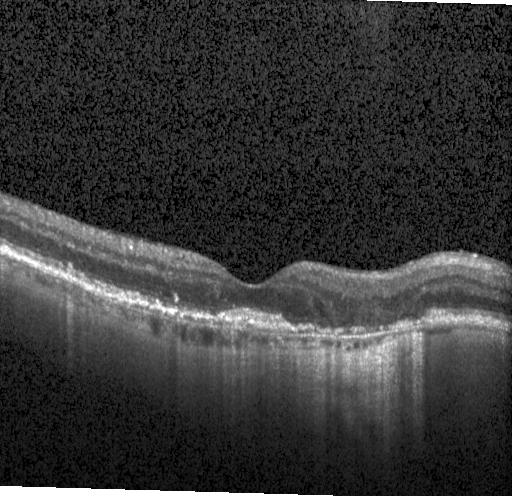 Spectral-domain OCT B-scan: choroidal neovascularization (CNV).